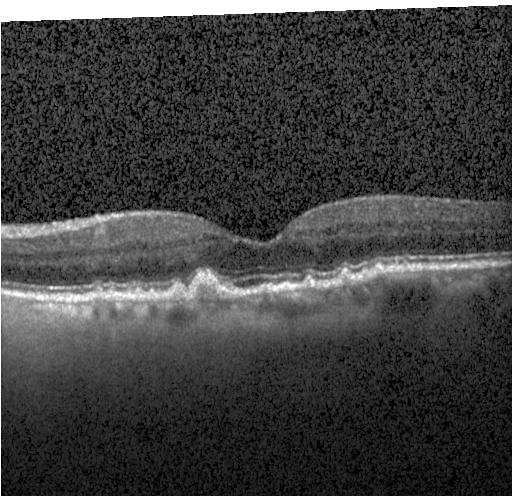 Macular OCT demonstrating sub-RPE drusenoid deposits.